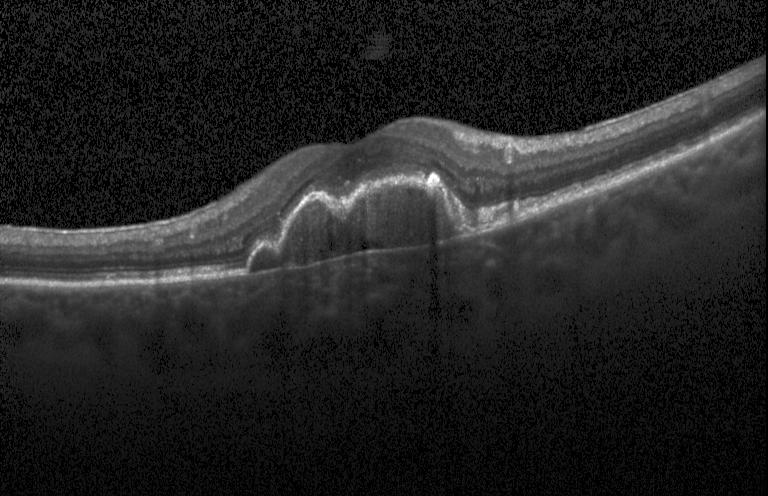

Optical coherence tomography B-scan. A choroidal neovascular membrane.